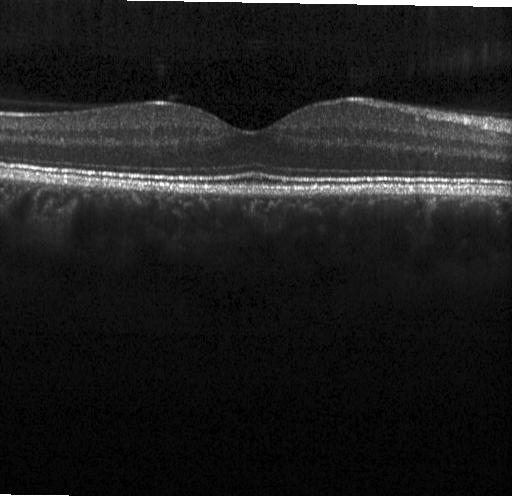 OCT B-scan; acquired on a Heidelberg Spectralis; centered on the fovea.
OCT finding: no choroidal neovascularization, no diabetic macular edema, and no drusen.